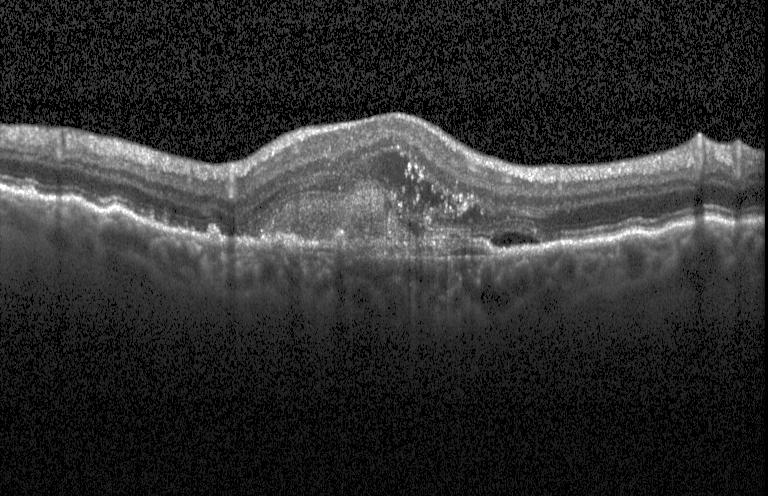

Instrument: Heidelberg Spectralis; spectral-domain OCT; through the macula; OCT line scan
Finding: a choroidal neovascular membrane.